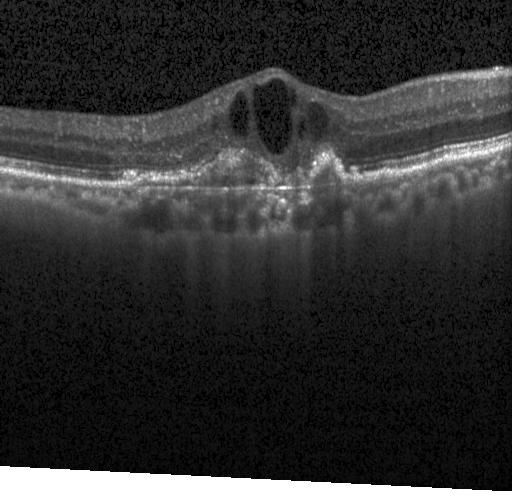 Retinal OCT cross-section. Fovea-centered.
Diagnosis: CNV.